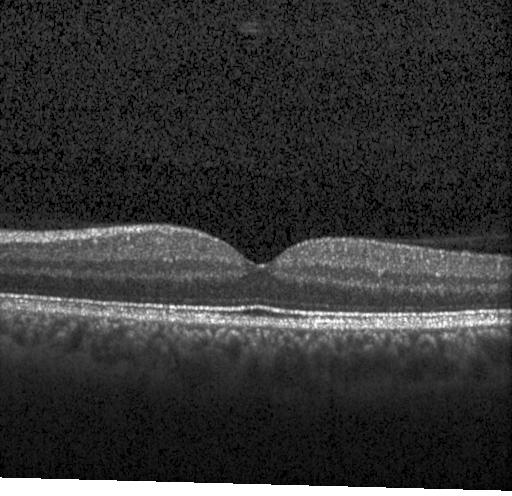 Impression: no choroidal neovascularization, diabetic macular edema, or drusen.